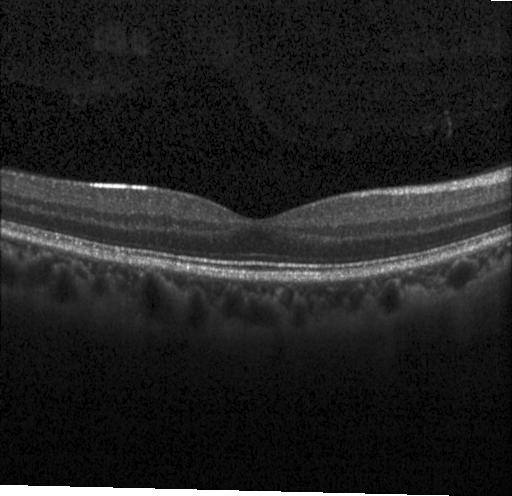 OCT B-scan showing no choroidal neovascularization, no diabetic macular edema, and no drusen.